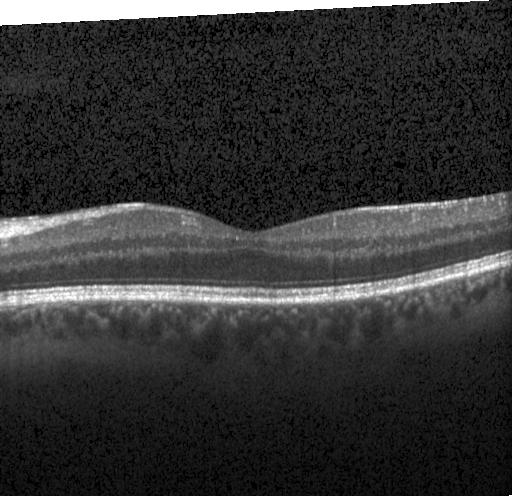

OCT finding: no evidence of choroidal neovascularization, diabetic macular edema, or drusen.